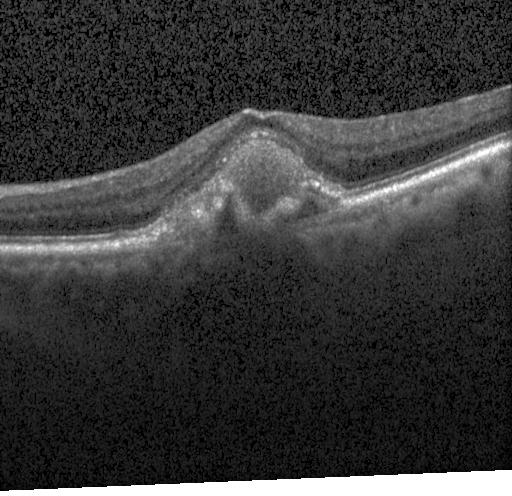
Spectral-domain OCT B-scan: CNV.